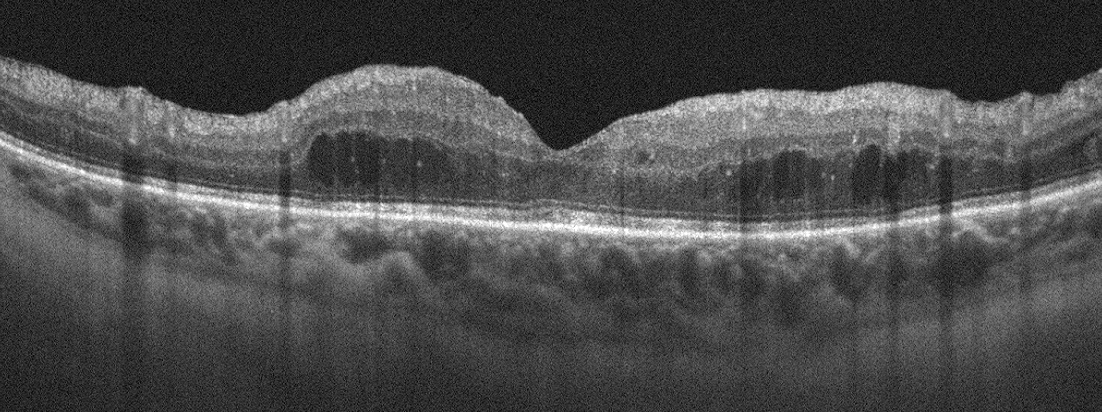
Retinal OCT B-scan.
Impression: DME.